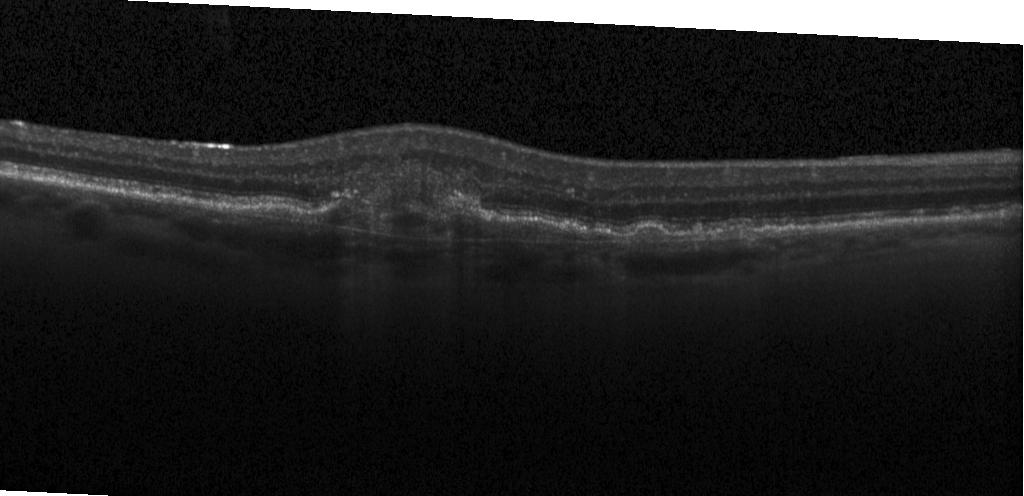
Spectral-domain optical coherence tomography · retinal OCT B-scan · Heidelberg Spectralis OCT system · horizontal scan through the fovea
Diagnosis: a choroidal neovascular membrane.